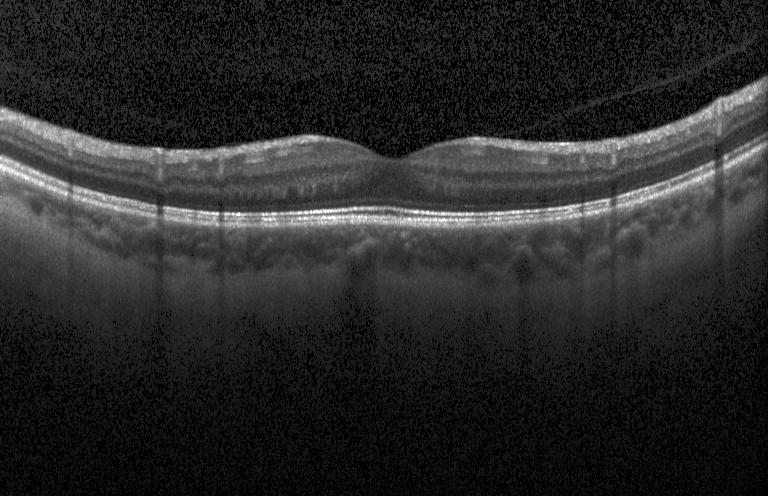
Retinal OCT cross-section · horizontal scan through the fovea · Heidelberg Spectralis OCT system · spectral-domain optical coherence tomography.
Finding: no evidence of CNV, DME, or drusen.